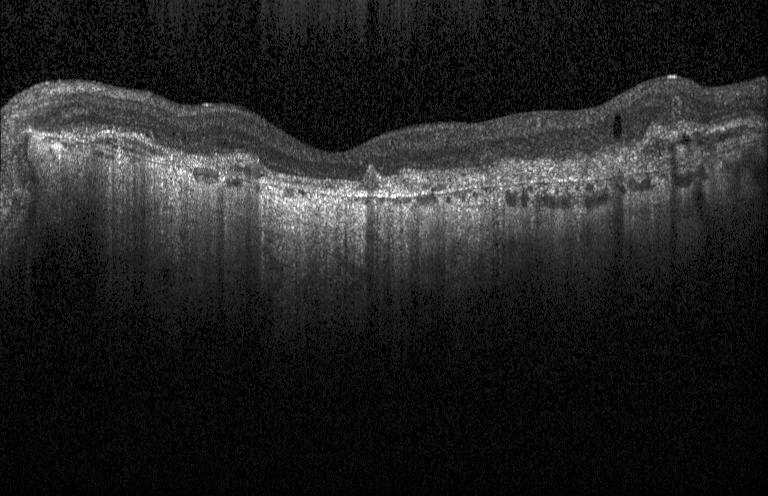 OCT B-scan — The scan shows choroidal neovascularization.